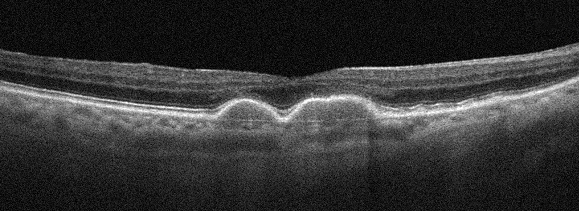 Optical coherence tomography B-scan, OD, acquired on an Optovue Avanti RTVue XR.
OCT finding: age-related macular degeneration (AMD).